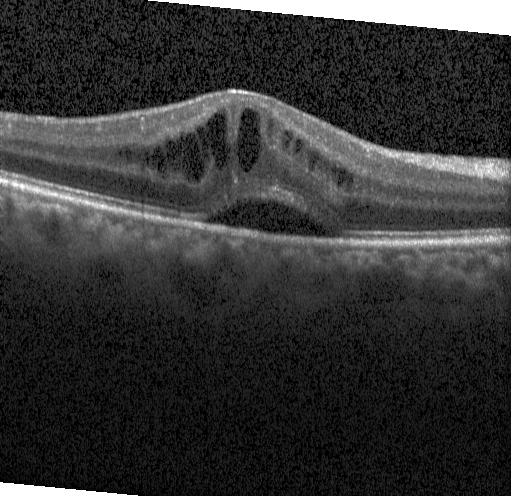
Macular scan · retinal OCT cross-section
Macular OCT: DME.